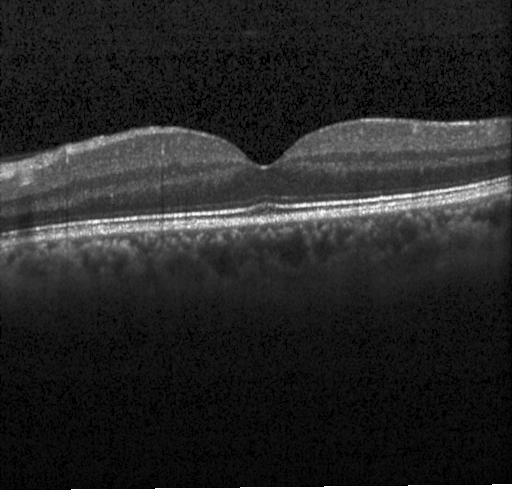

OCT scan showing no evidence of choroidal neovascularization, diabetic macular edema, or drusen.